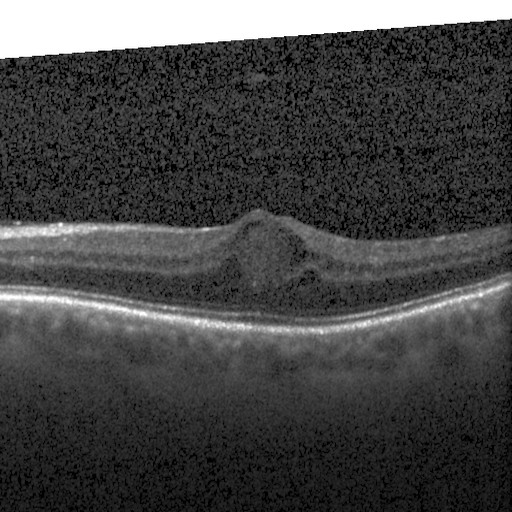

OCT scan showing diabetic macular edema (DME).